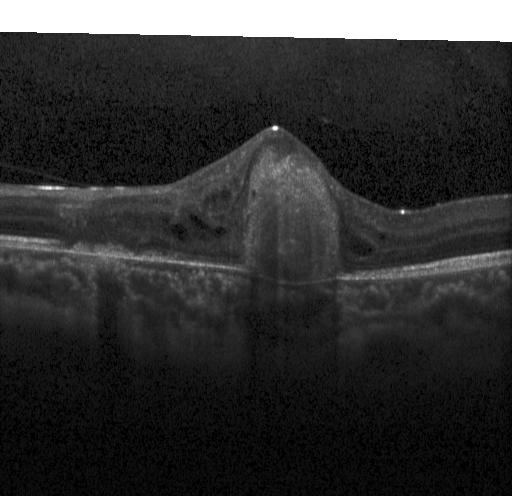

OCT line scan
Diagnosis: a choroidal neovascular membrane.